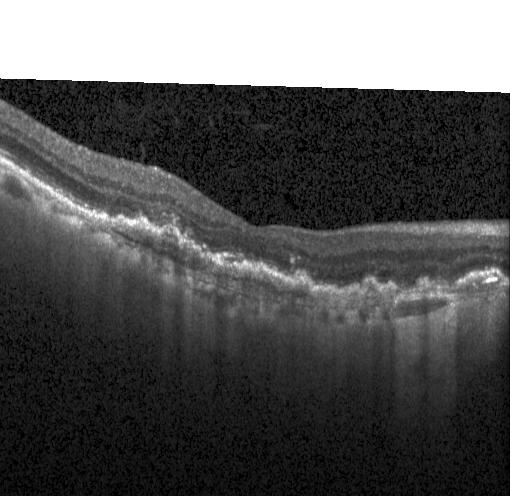 Retinal OCT B-scan · instrument: Heidelberg Spectralis · centered on the fovea. OCT finding: choroidal neovascularization (CNV).